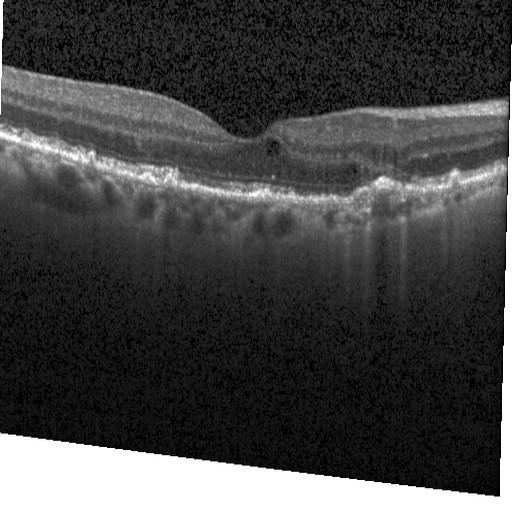

Retinal OCT B-scan; SD-OCT; horizontal scan through the fovea. This B-scan demonstrates diabetic macular edema (DME).